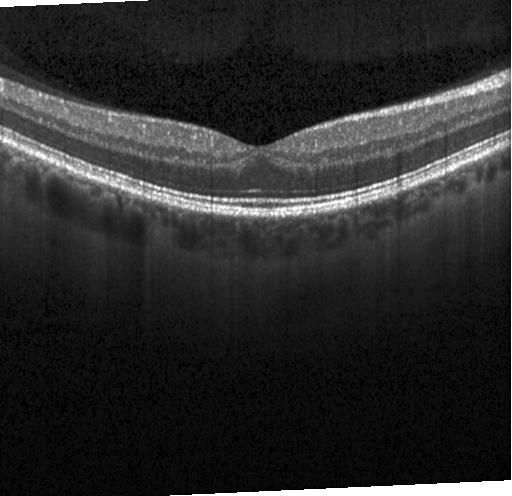
Optical coherence tomography scan; Heidelberg Spectralis OCT system; macular scan. Dx: no evidence of CNV, DME, or drusen.